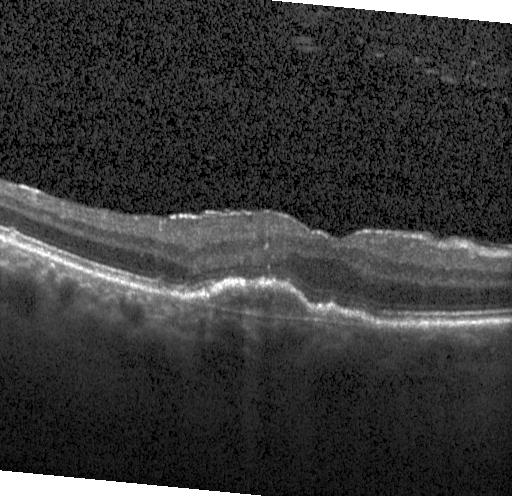 Finding: a choroidal neovascular membrane.